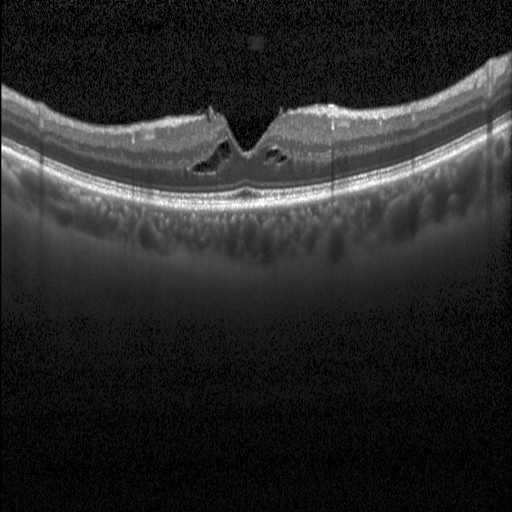

Retinal OCT B-scan.
Diagnosis: diabetic macular edema.